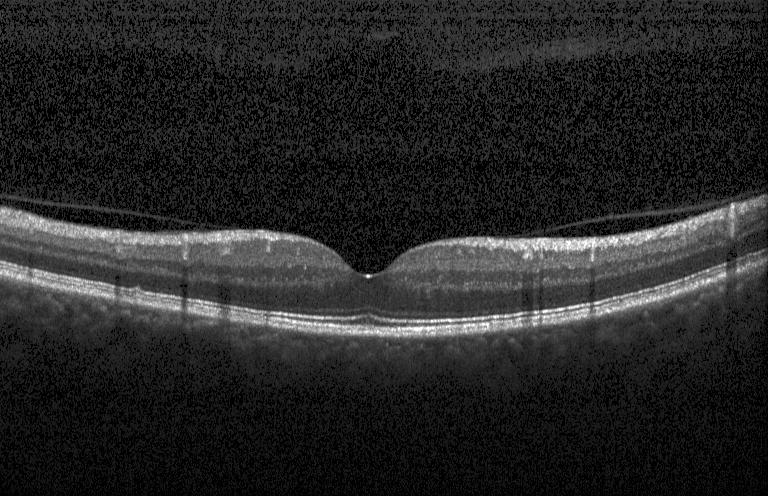 OCT scan showing no CNV, DME, or drusen.